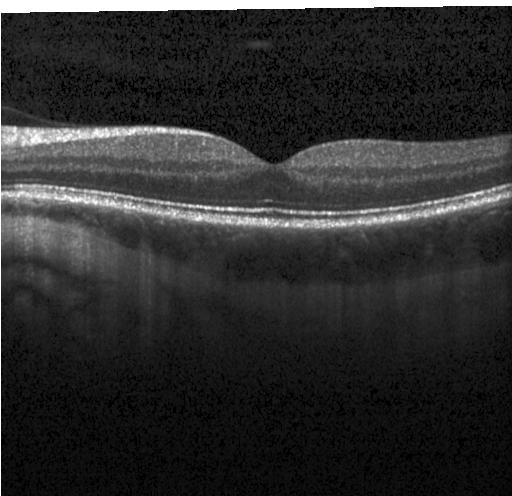

OCT scan showing no evidence of choroidal neovascularization, diabetic macular edema, or drusen.